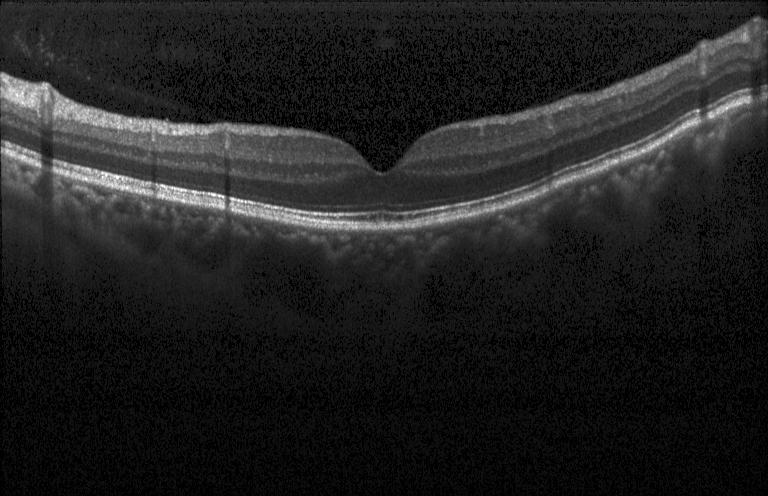 OCT B-scan · instrument: Heidelberg Spectralis · macular scan. Macular OCT: neither CNV, DME, nor drusen.